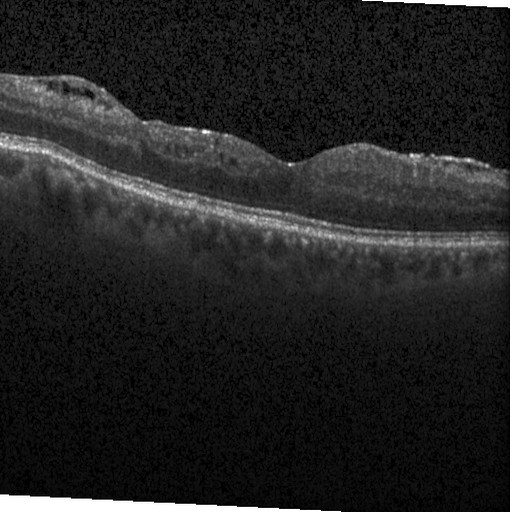 OCT line scan — Impression: diabetic macular edema (DME).